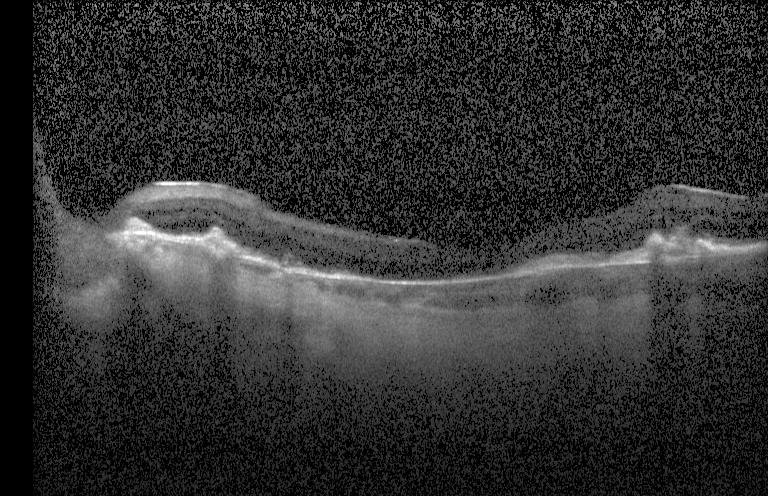
Through the macula, spectral-domain optical coherence tomography, acquired on a Heidelberg Spectralis, optical coherence tomography scan.
OCT finding: a choroidal neovascular membrane.